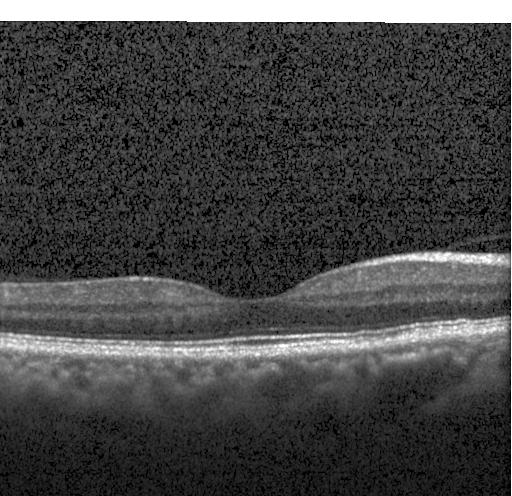 Macular scan. Retinal OCT cross-section. Heidelberg Spectralis — No choroidal neovascularization, no diabetic macular edema, and no drusen.